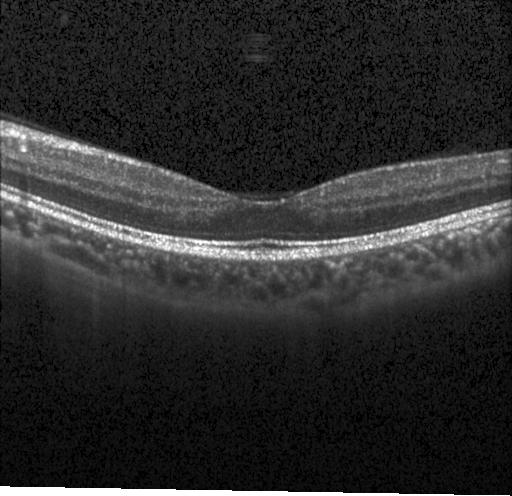

Fovea-centered · Heidelberg Spectralis · spectral-domain optical coherence tomography · OCT B-scan
This B-scan demonstrates no CNV, no DME, and no drusen.